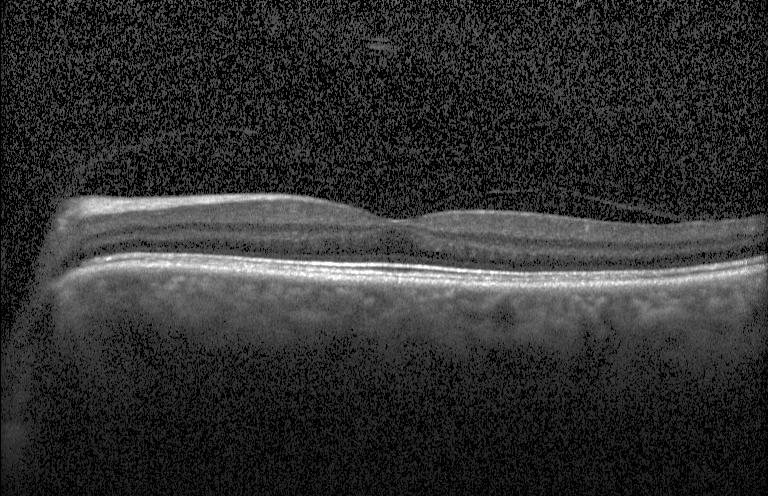

Heidelberg Spectralis, retinal OCT B-scan. The scan shows no evidence of choroidal neovascularization, diabetic macular edema, or drusen.